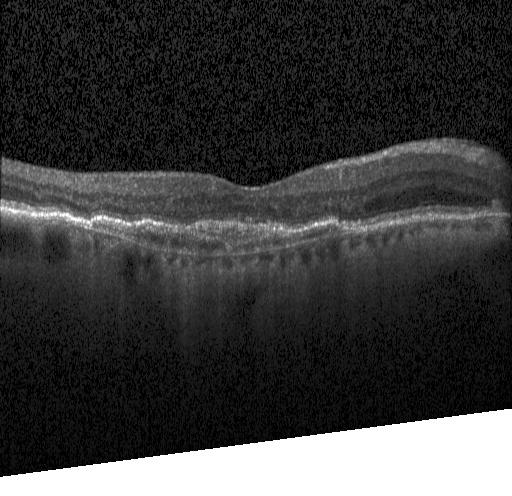

Spectral-domain optical coherence tomography, centered on the fovea, OCT B-scan, Heidelberg Spectralis — Diagnosis: a choroidal neovascular membrane.